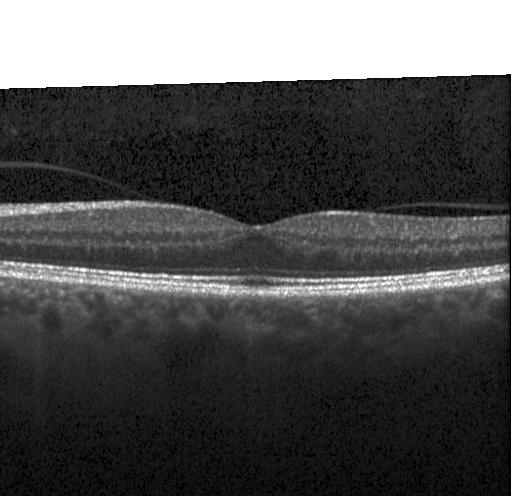
Retinal OCT cross-section; instrument: Heidelberg Spectralis; SD-OCT.
Impression: no CNV, DME, or drusen.